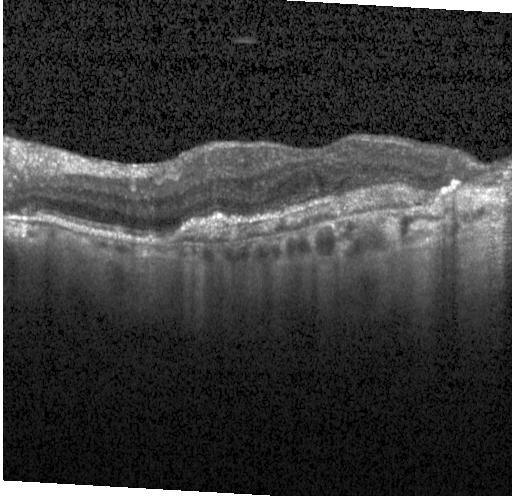
The scan shows a choroidal neovascular membrane.